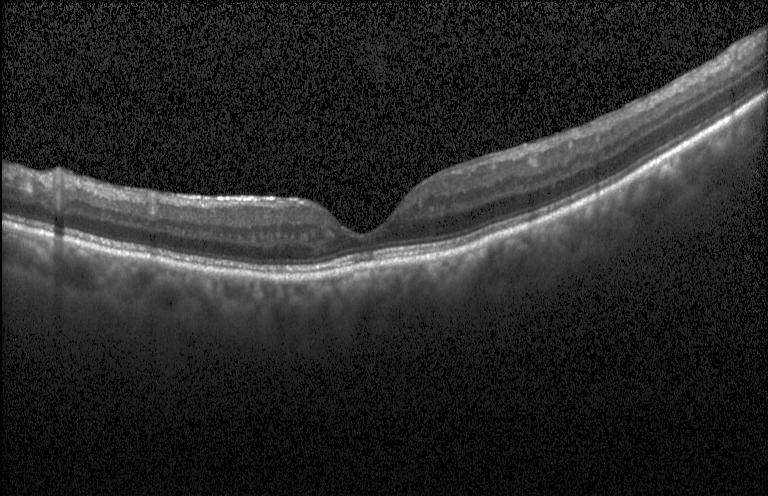

No choroidal neovascularization, diabetic macular edema, or drusen.